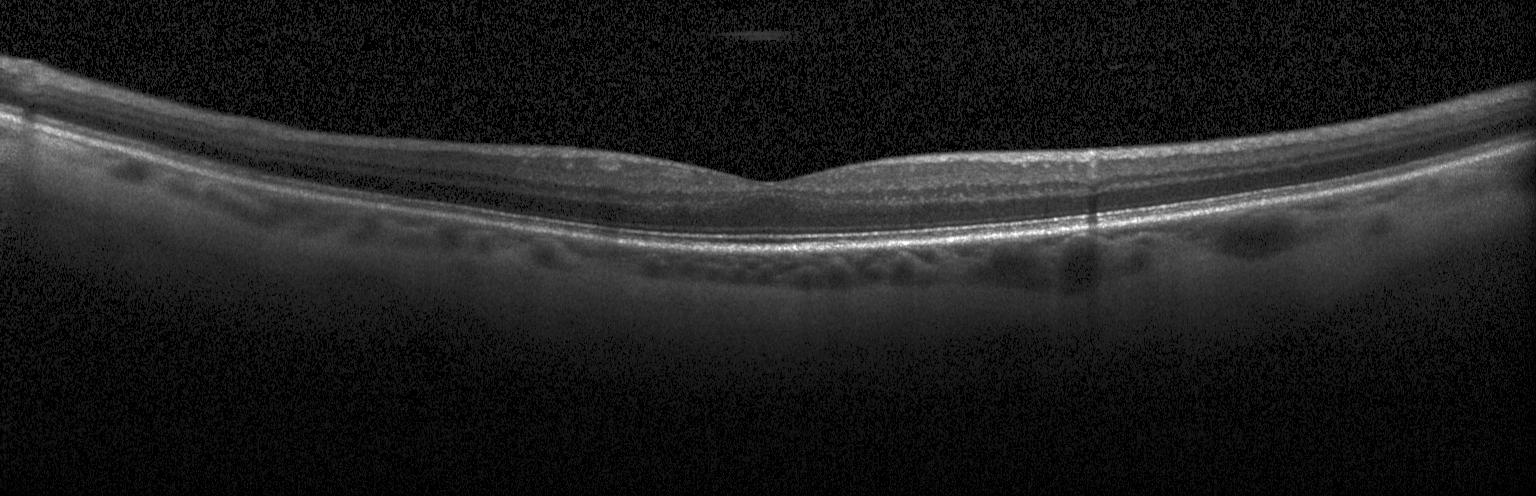
SD-OCT · instrument: Heidelberg Spectralis · fovea-centered · OCT line scan — Assessment: no choroidal neovascularization, diabetic macular edema, or drusen.